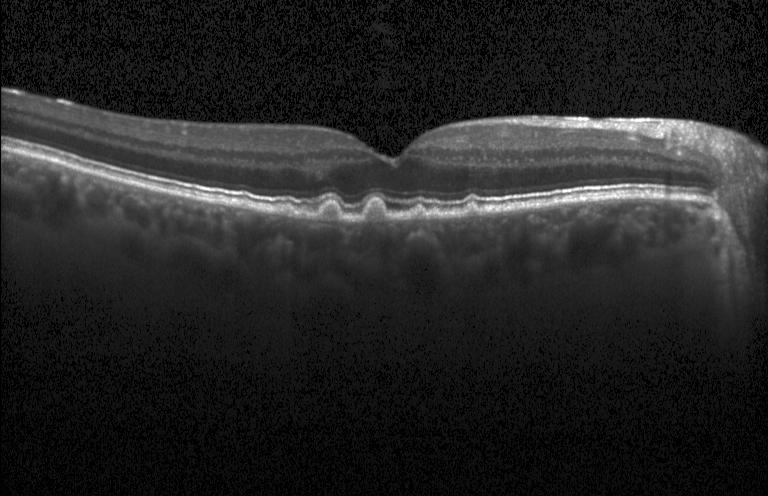 Optical coherence tomography B-scan.
Assessment: drusen.